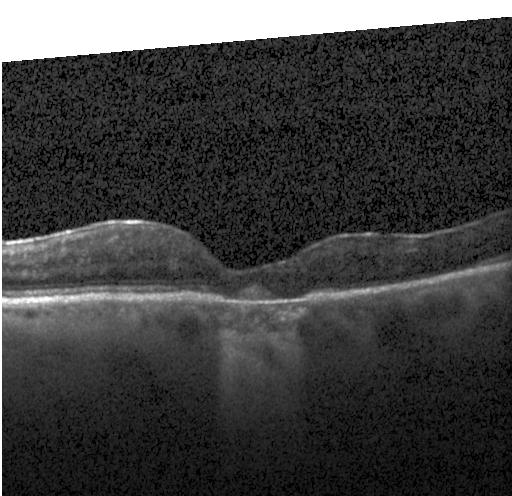 Retinal OCT cross-section, acquired on a Heidelberg Spectralis, horizontal scan through the fovea. The scan shows choroidal neovascularization.